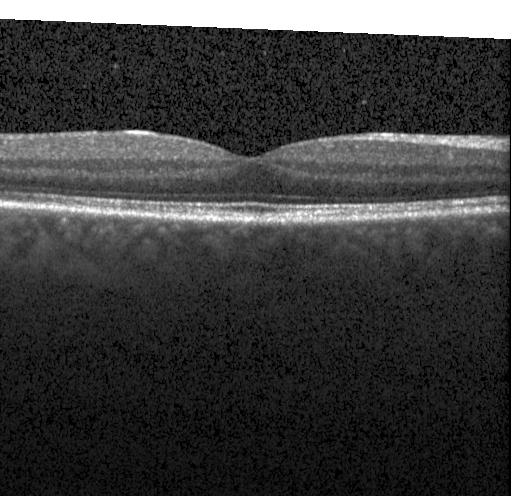
Macular scan; spectral-domain optical coherence tomography; acquired on a Heidelberg Spectralis; retinal OCT B-scan
Dx: no choroidal neovascularization, diabetic macular edema, or drusen.